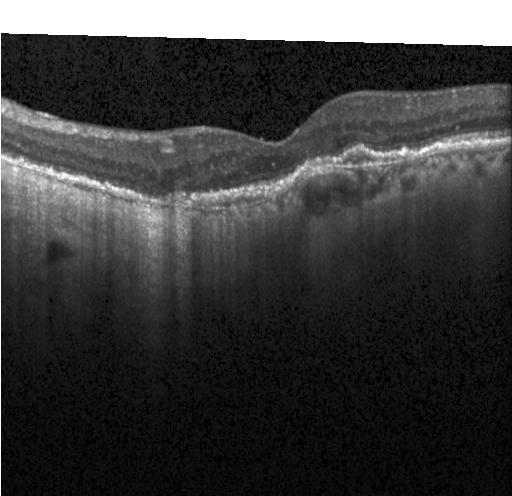
Retinal OCT cross-section — OCT finding: choroidal neovascularization (CNV).